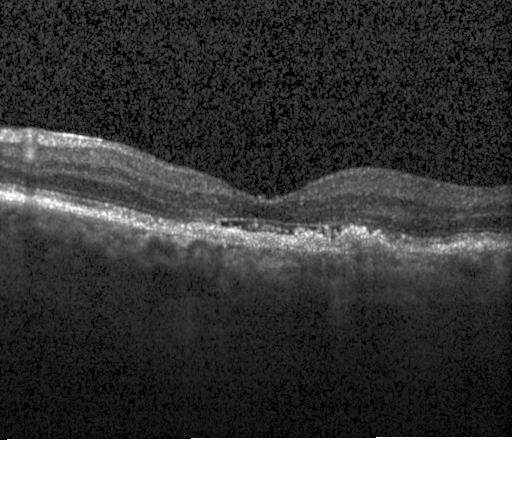 Centered on the fovea · spectral-domain optical coherence tomography · OCT line scan · Heidelberg Spectralis.
Choroidal neovascularization (CNV).